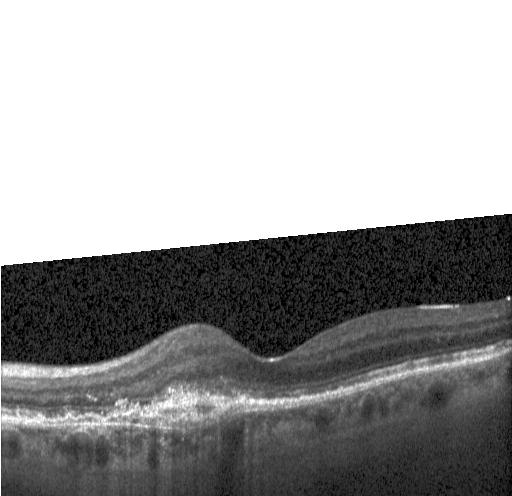
The scan shows a choroidal neovascular membrane.